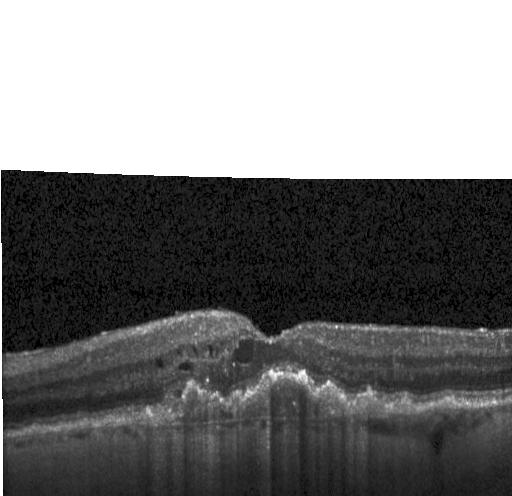
Impression: a choroidal neovascular membrane.